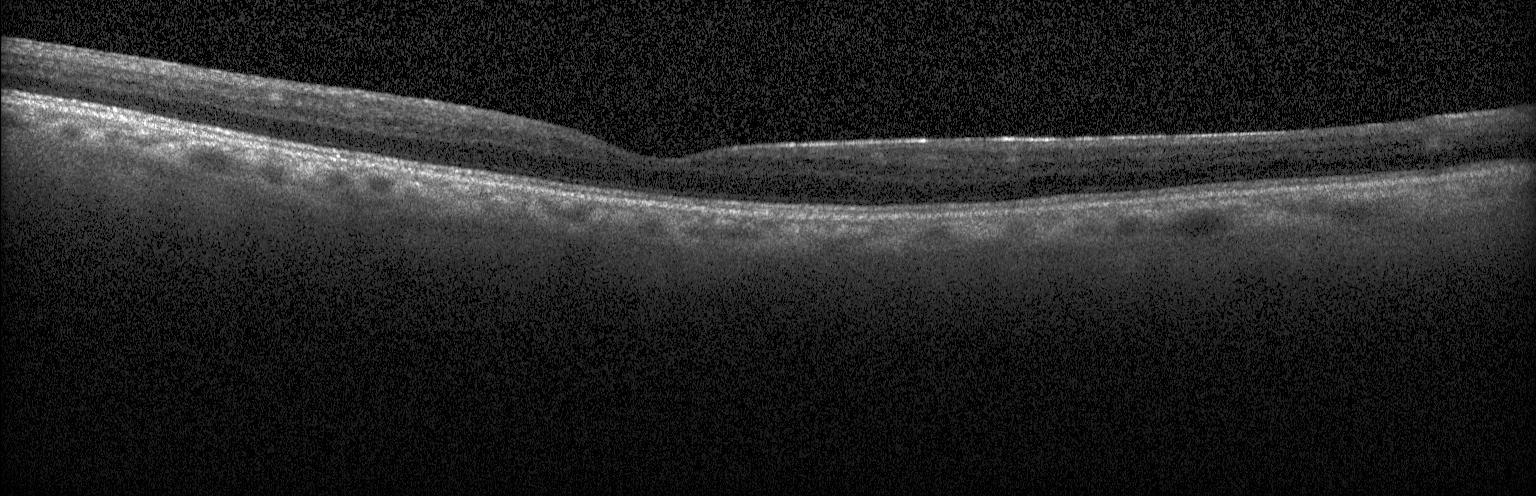

Dx: no evidence of choroidal neovascularization, diabetic macular edema, or drusen.